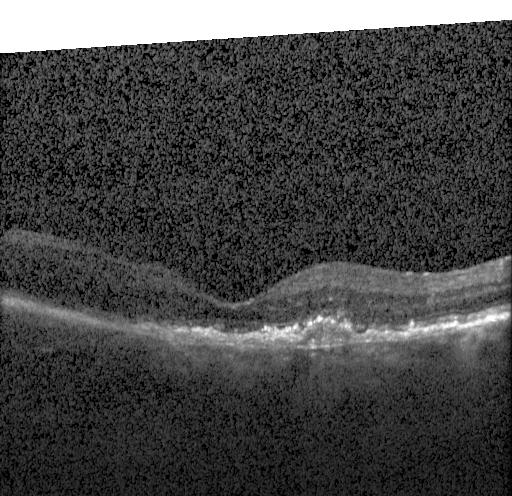 The scan shows a choroidal neovascular membrane.